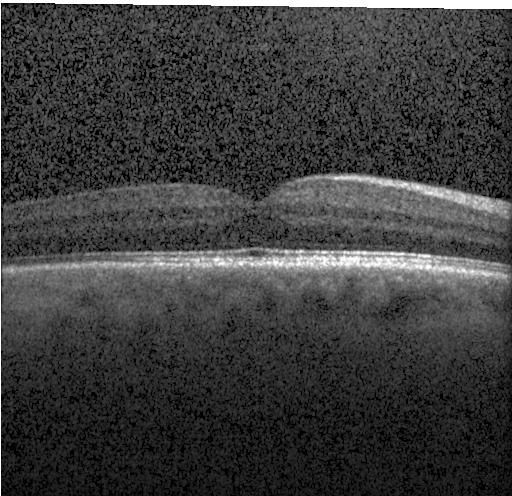

Optical coherence tomography B-scan. Fovea-centered. Finding: no choroidal neovascularization, no diabetic macular edema, and no drusen.